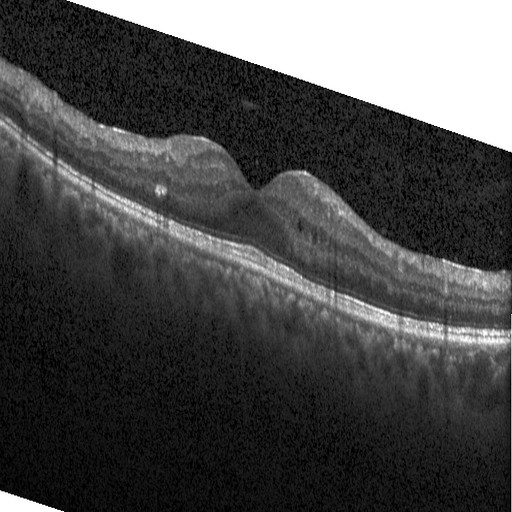

Spectral-domain OCT B-scan: DME.